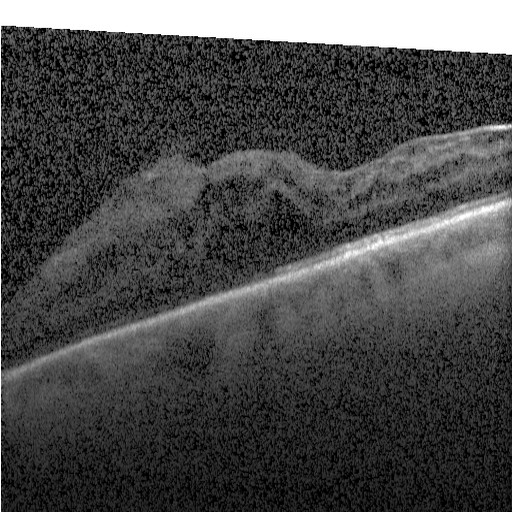

Spectral-domain OCT. Optical coherence tomography B-scan. Instrument: Heidelberg Spectralis
Assessment: diabetic macular edema (DME).